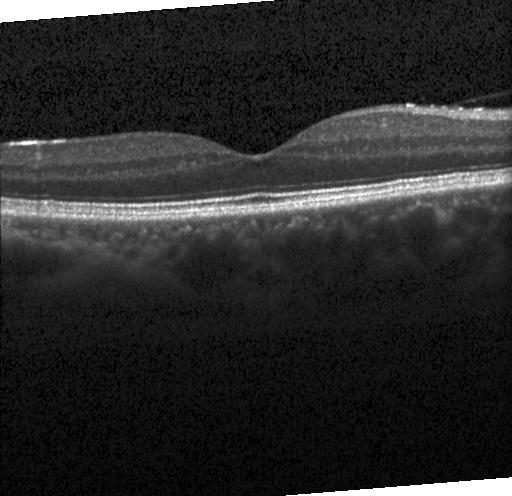
Retinal OCT B-scan, Heidelberg Spectralis.
OCT finding: neither choroidal neovascularization, diabetic macular edema, nor drusen.